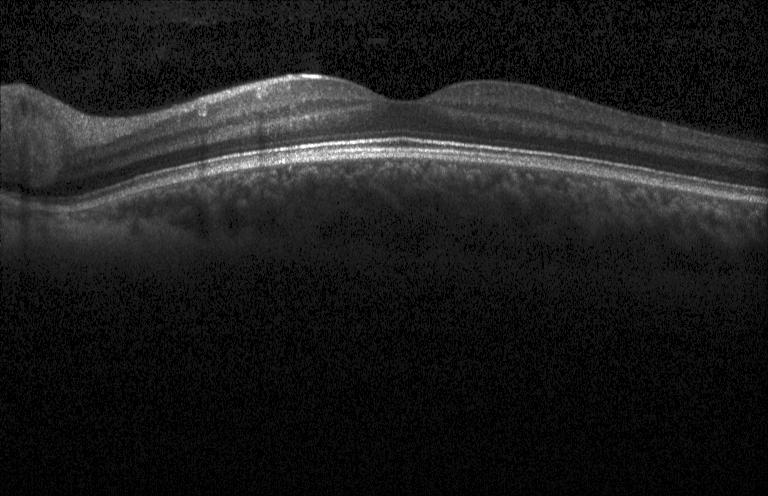

Finding: neither choroidal neovascularization, diabetic macular edema, nor drusen.